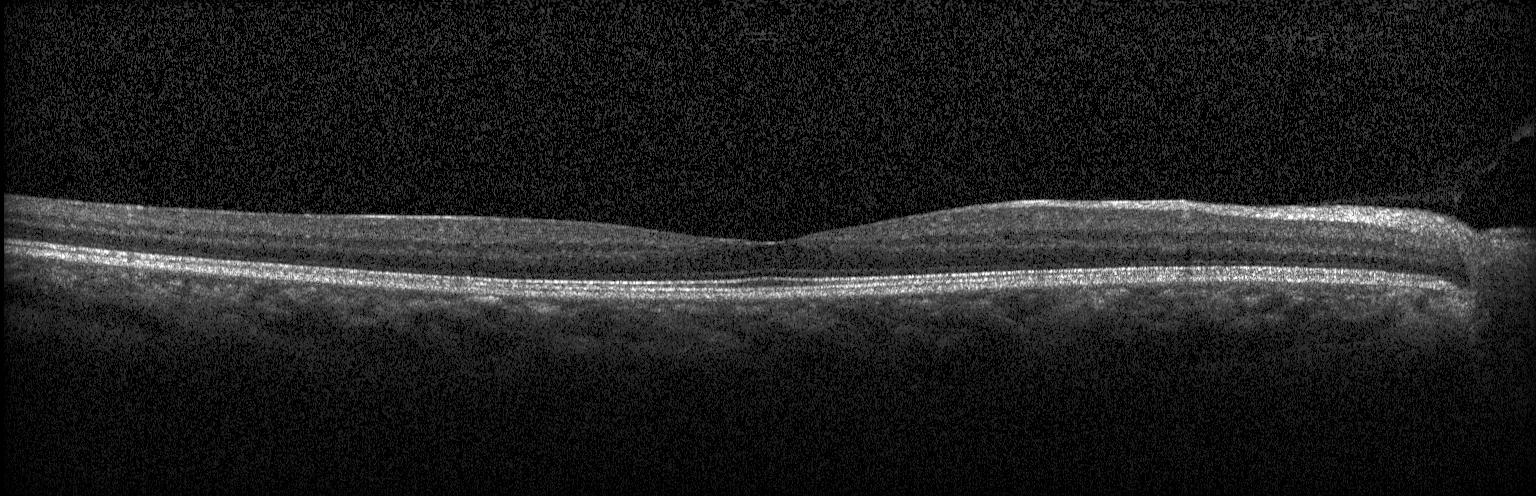
Optical coherence tomography B-scan, Heidelberg Spectralis. Impression: no choroidal neovascularization, diabetic macular edema, or drusen.